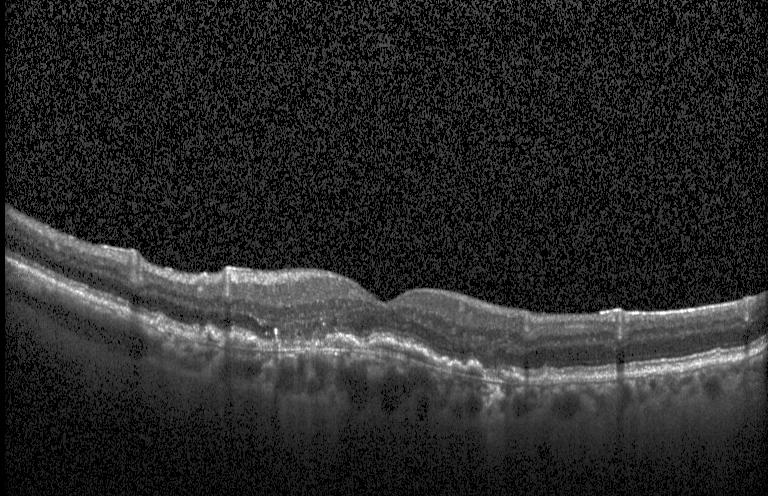
Optical coherence tomography scan · Heidelberg Spectralis
Assessment: a choroidal neovascular membrane.